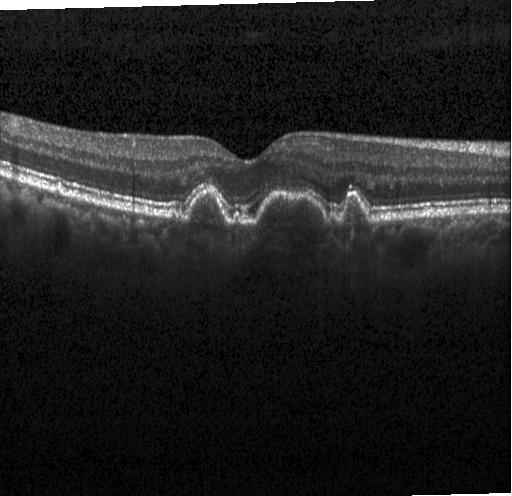

Retinal OCT B-scan — This B-scan demonstrates multiple drusen.